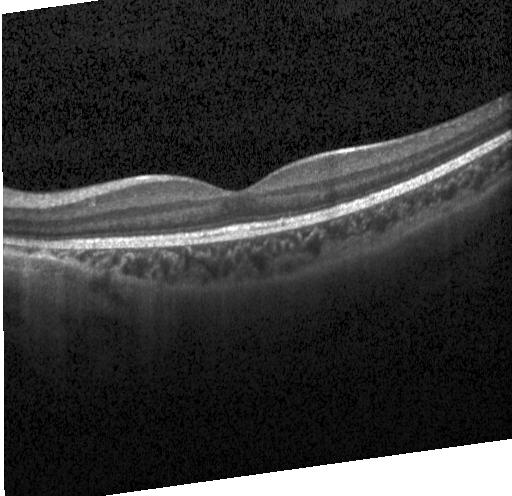
Retinal OCT cross-section · spectral-domain OCT. Diagnosis: no choroidal neovascularization, diabetic macular edema, or drusen.